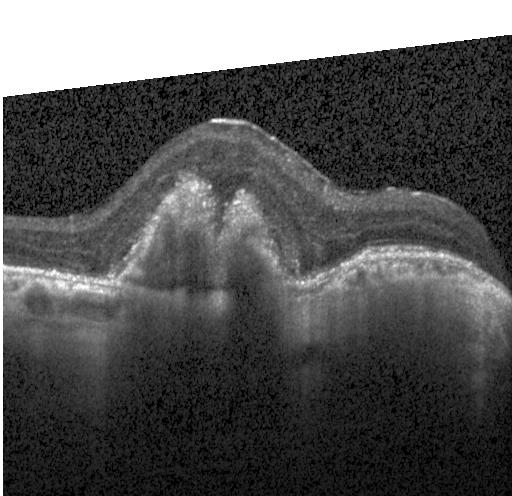
Retinal OCT cross-section showing a choroidal neovascular membrane.